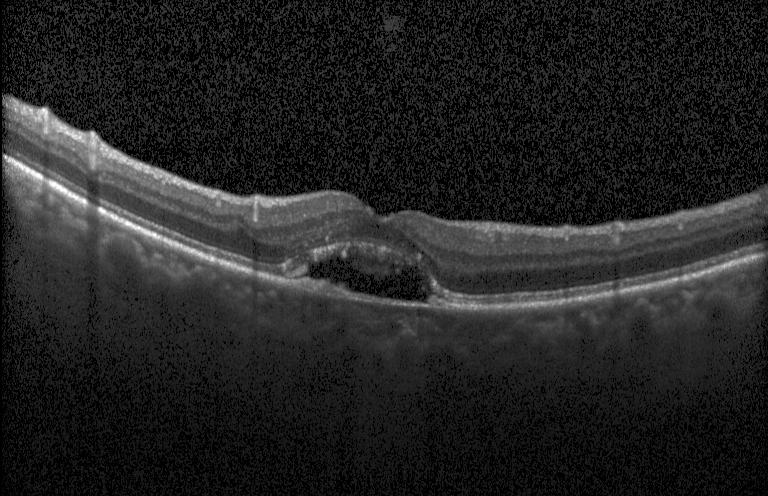
Optical coherence tomography B-scan; Heidelberg Spectralis; horizontal scan through the fovea.
OCT finding: choroidal neovascularization.